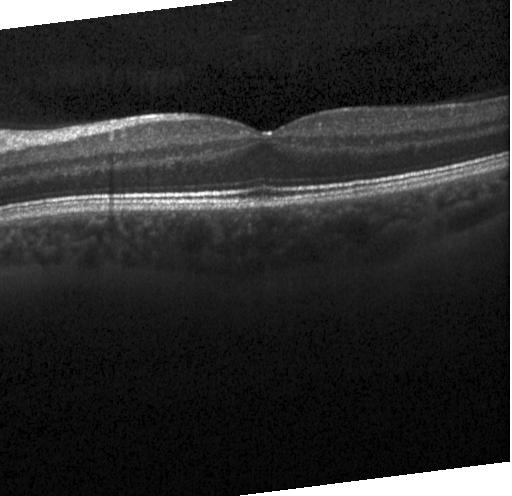

OCT line scan. The scan shows no choroidal neovascularization, diabetic macular edema, or drusen.